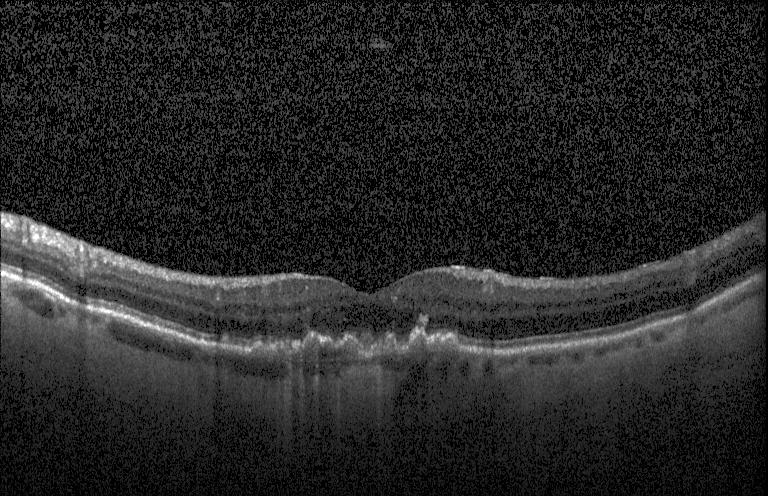
Macular scan, instrument: Heidelberg Spectralis, optical coherence tomography scan.
Macular OCT: sub-RPE drusenoid deposits.